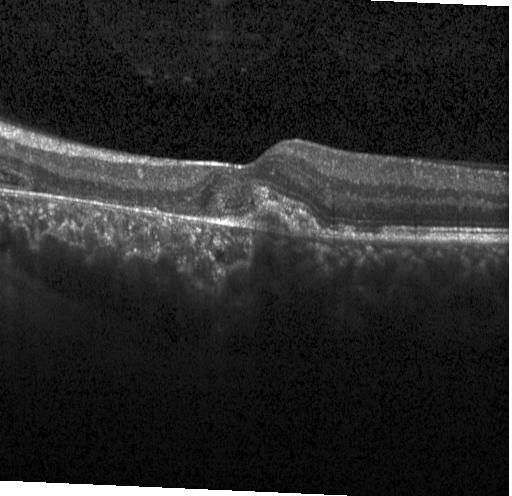 Centered on the fovea. Optical coherence tomography B-scan
Diagnosis: a choroidal neovascular membrane.